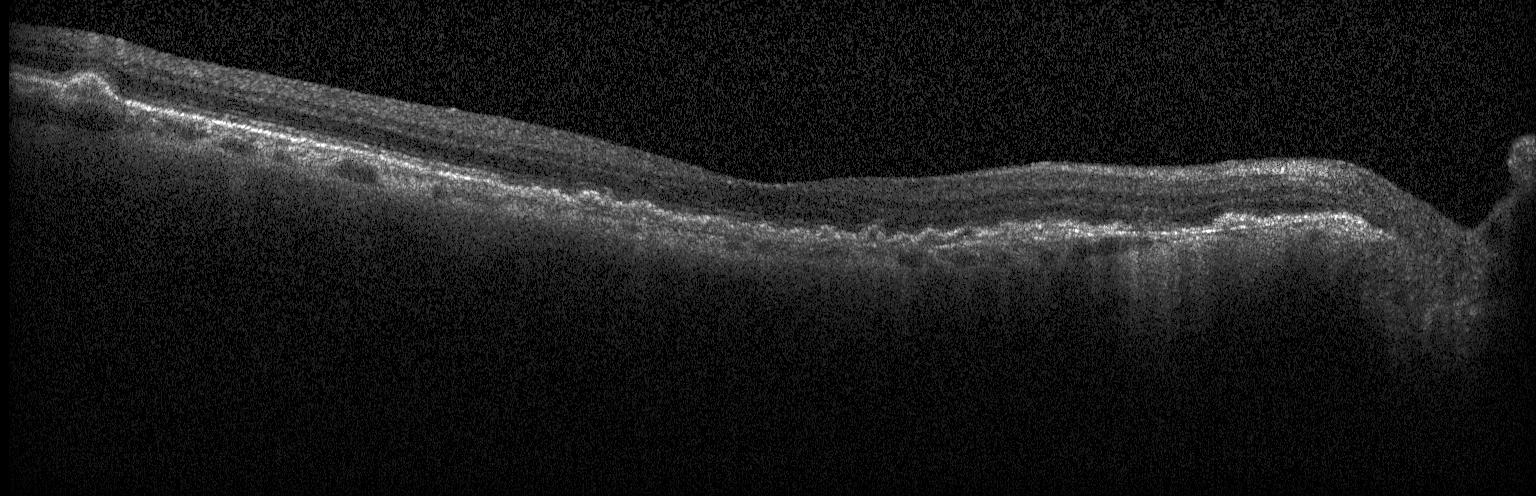 Macular OCT demonstrating choroidal neovascularization (CNV).